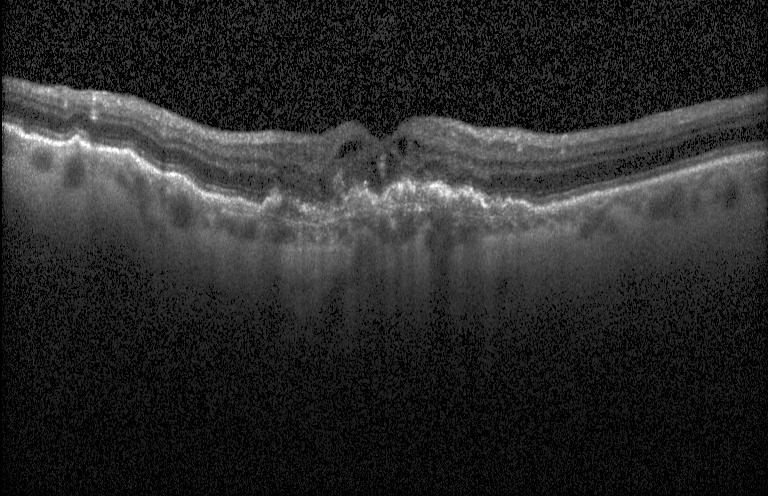

Acquired on a Heidelberg Spectralis; fovea-centered; spectral-domain OCT; retinal OCT cross-section. Diagnosis: a choroidal neovascular membrane.